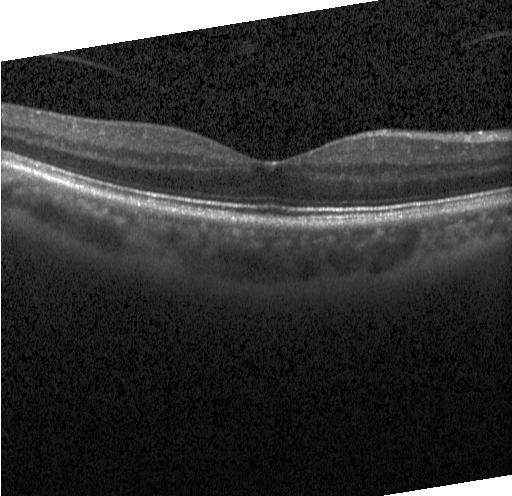 Macular OCT: no evidence of choroidal neovascularization, diabetic macular edema, or drusen.